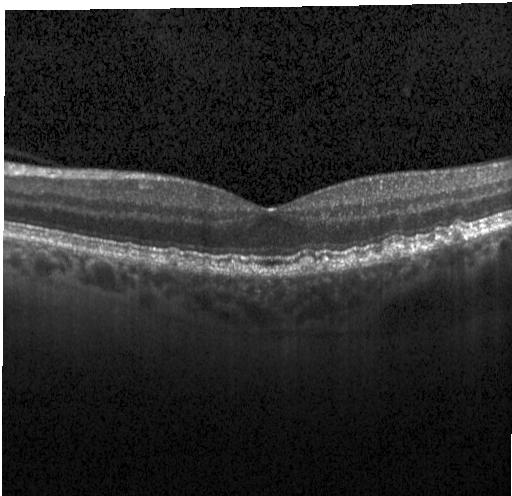
Impression: multiple drusen.